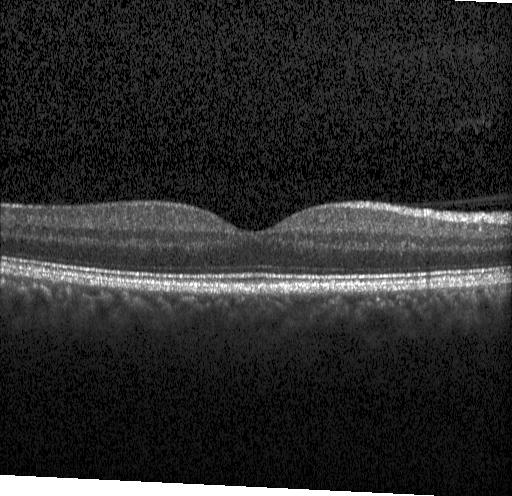

No choroidal neovascularization, diabetic macular edema, or drusen.